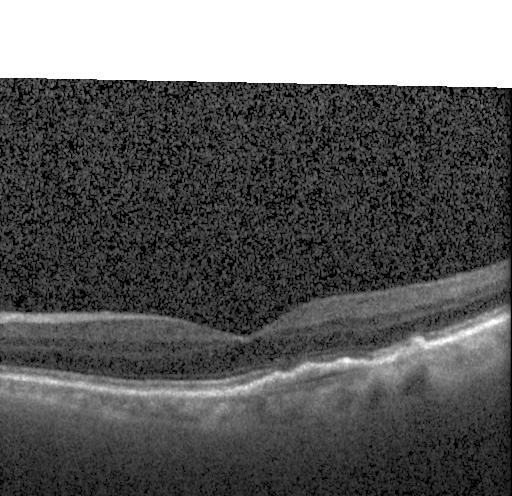

OCT scan showing a choroidal neovascular membrane.